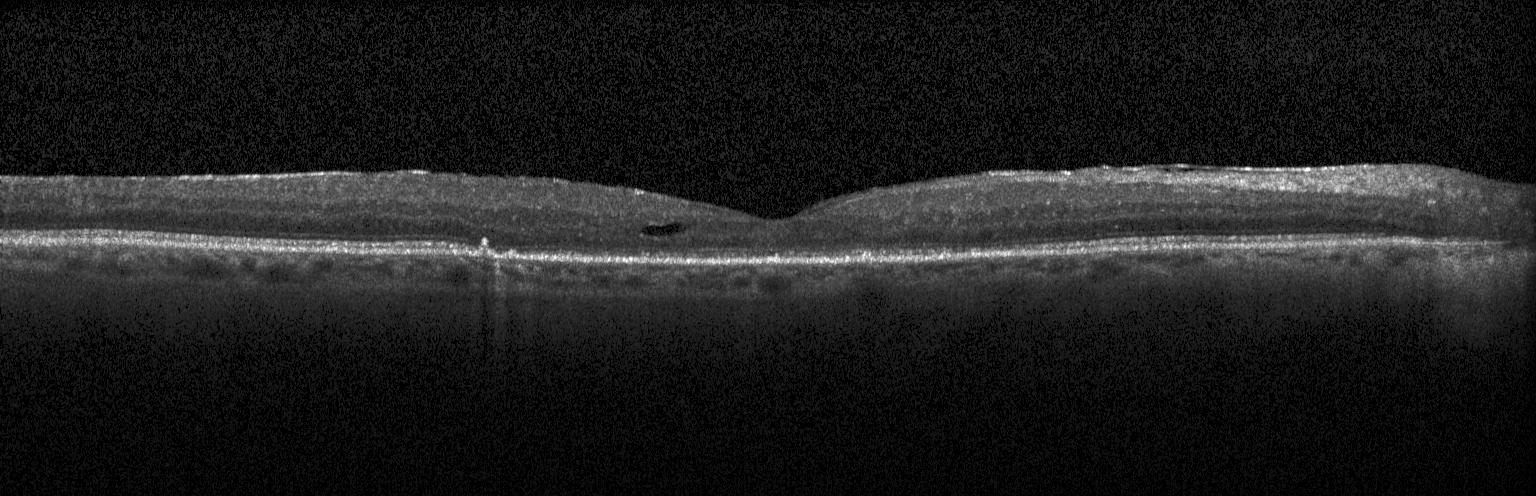
Macular scan. Optical coherence tomography scan. Spectral-domain OCT
Finding: diabetic macular edema (DME).